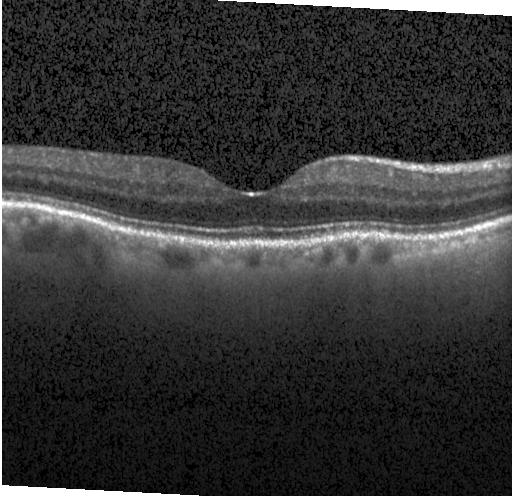

OCT B-scan.
OCT finding: neither CNV, DME, nor drusen.